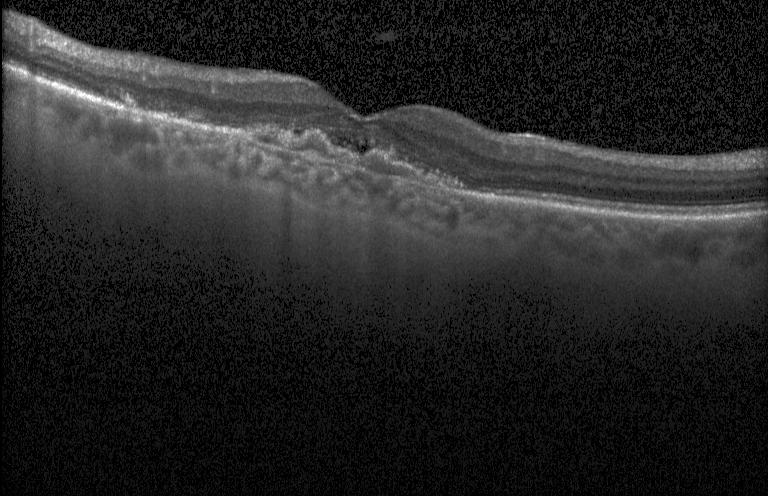 Instrument: Heidelberg Spectralis. Retinal OCT B-scan.
Macular OCT: choroidal neovascularization (CNV).